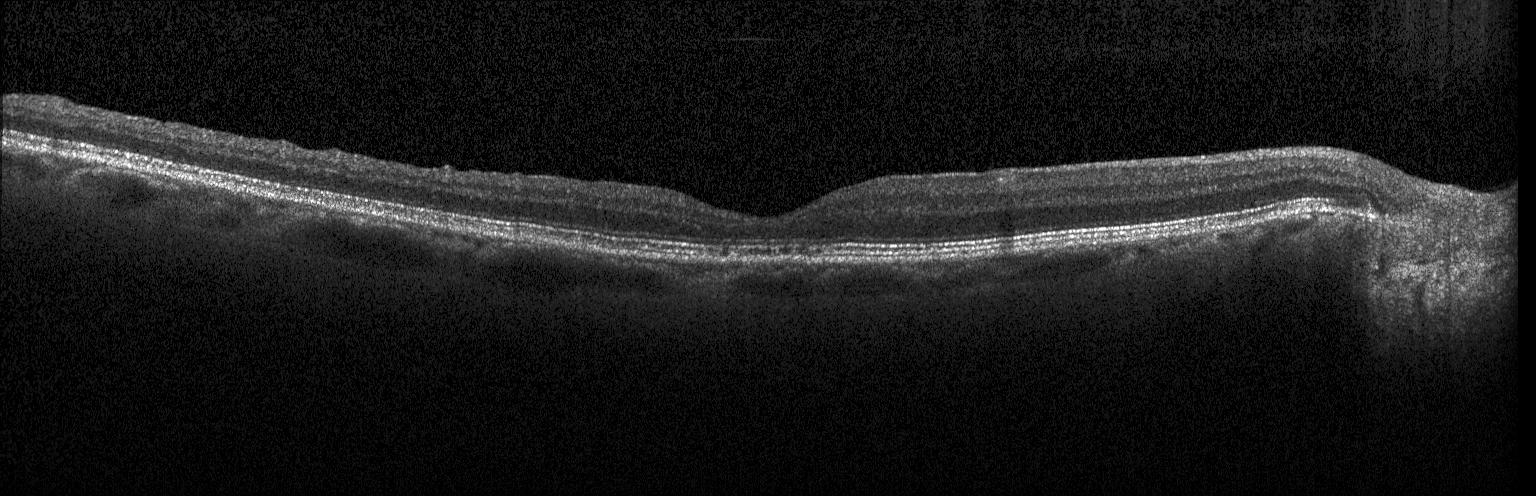 Through the macula; Heidelberg Spectralis OCT system; spectral-domain optical coherence tomography; retinal OCT B-scan — This B-scan demonstrates no evidence of choroidal neovascularization, diabetic macular edema, or drusen.